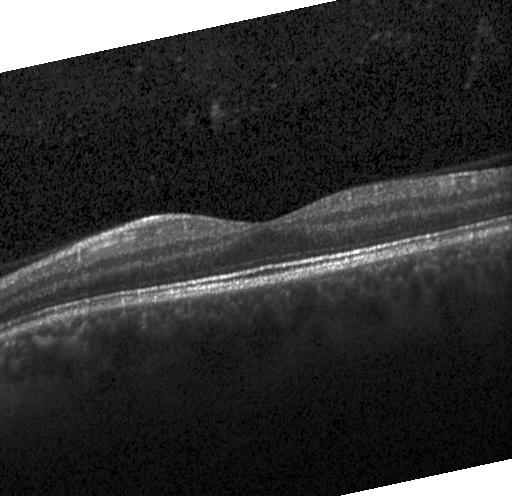 Optical coherence tomography scan, instrument: Heidelberg Spectralis, horizontal scan through the fovea
No choroidal neovascularization, diabetic macular edema, or drusen.